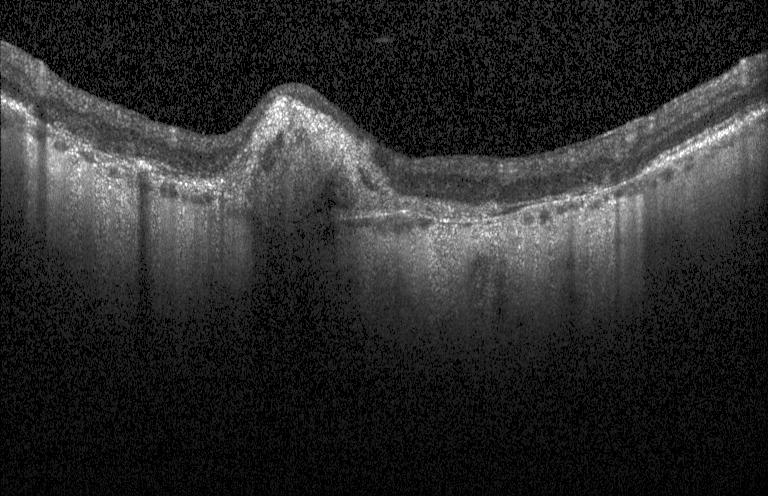

Impression: choroidal neovascularization (CNV).